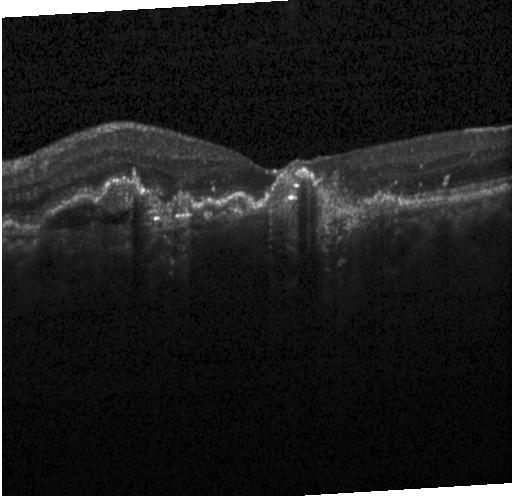 Assessment: CNV.